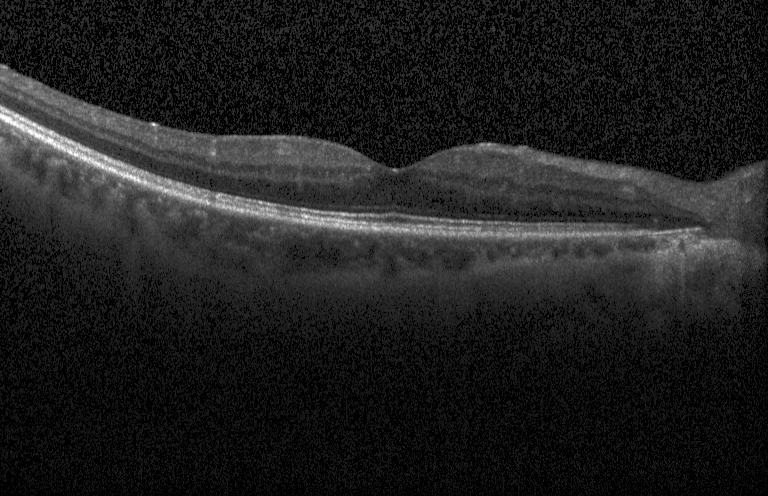

Optical coherence tomography scan
Diagnosis: neither choroidal neovascularization, diabetic macular edema, nor drusen.